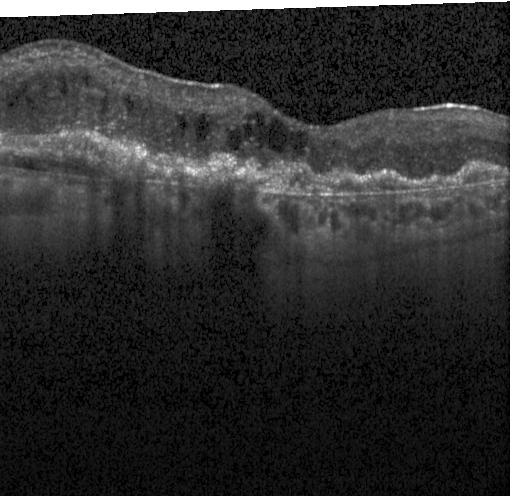 Macular OCT: choroidal neovascularization (CNV).